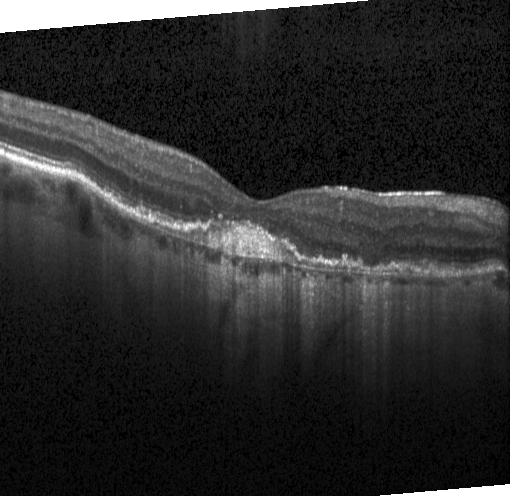 Heidelberg Spectralis OCT system. Macular scan. Retinal OCT B-scan
Diagnosis: a choroidal neovascular membrane.